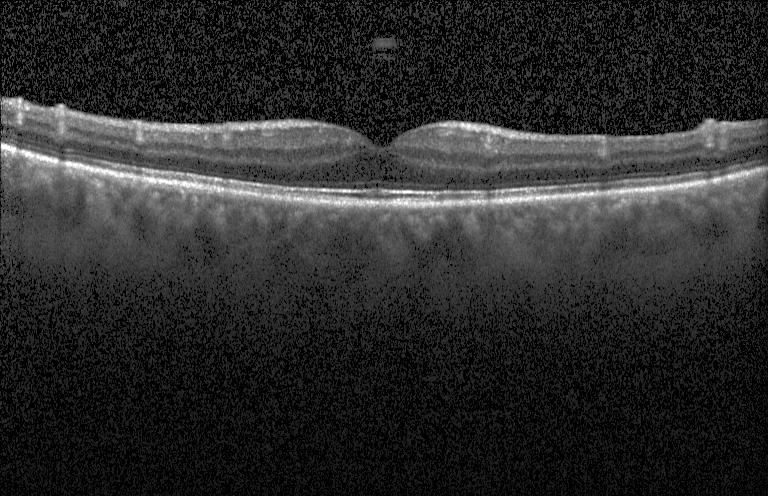

OCT line scan; macular scan; instrument: Heidelberg Spectralis. Diagnosis: no CNV, DME, or drusen.